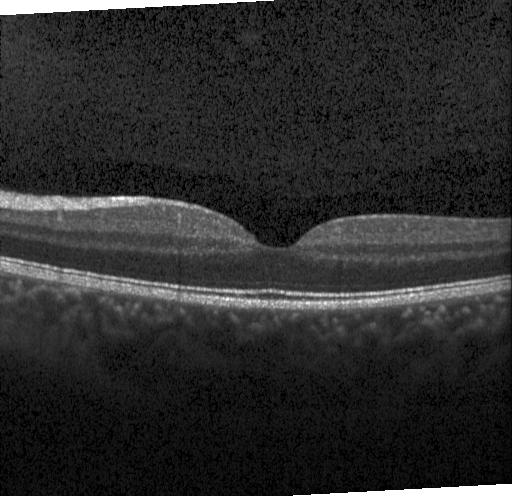

Spectral-domain OCT B-scan: no CNV, no DME, and no drusen.